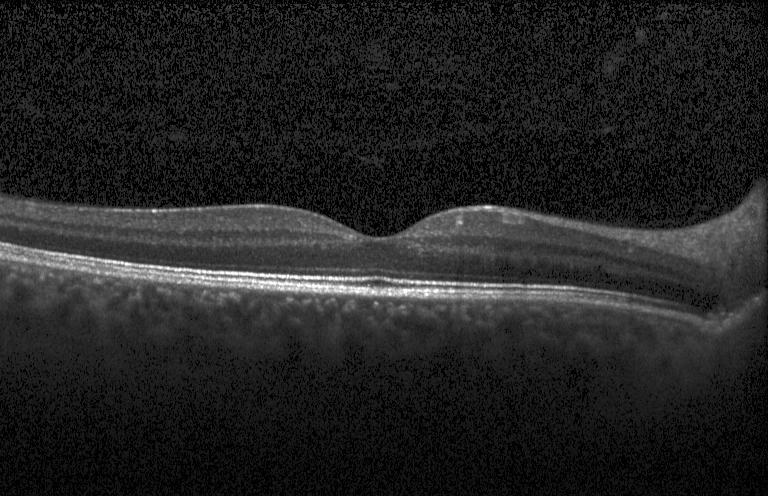 Optical coherence tomography B-scan
The scan shows neither choroidal neovascularization, diabetic macular edema, nor drusen.